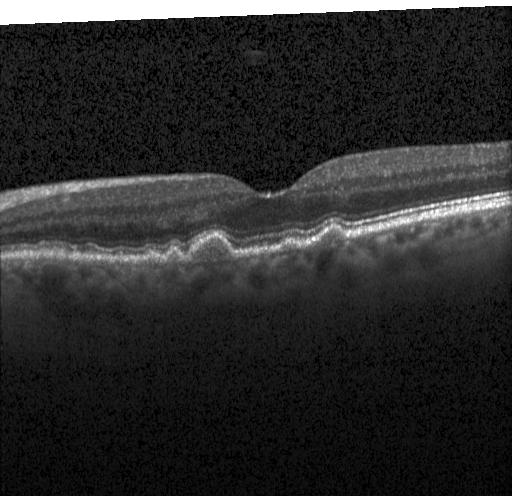
Spectral-domain optical coherence tomography · fovea-centered · Heidelberg Spectralis OCT system · optical coherence tomography B-scan
Finding: sub-RPE drusenoid deposits.